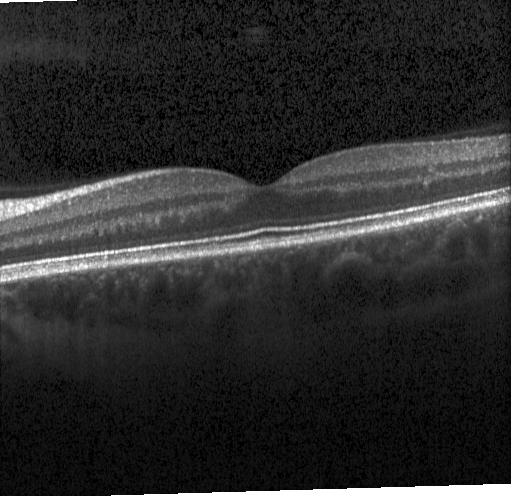
Finding: no choroidal neovascularization, diabetic macular edema, or drusen.